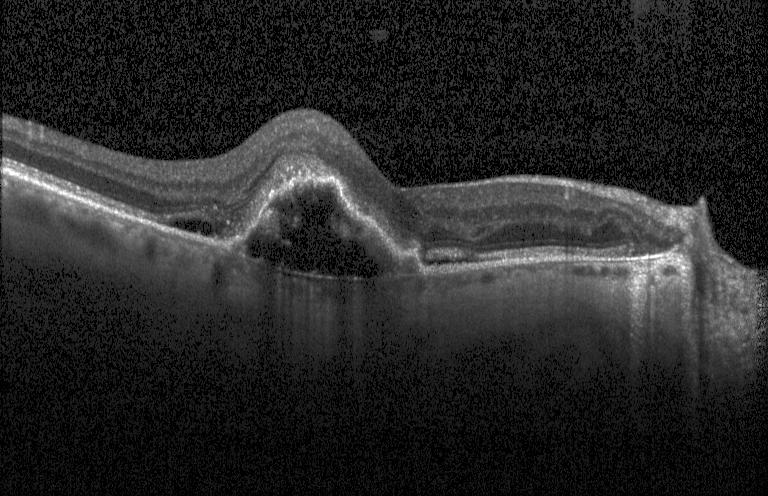
Assessment: a choroidal neovascular membrane.